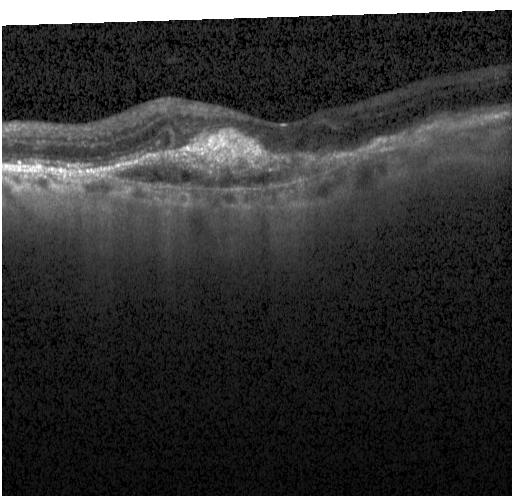 Instrument: Heidelberg Spectralis · optical coherence tomography B-scan — The scan shows a choroidal neovascular membrane.